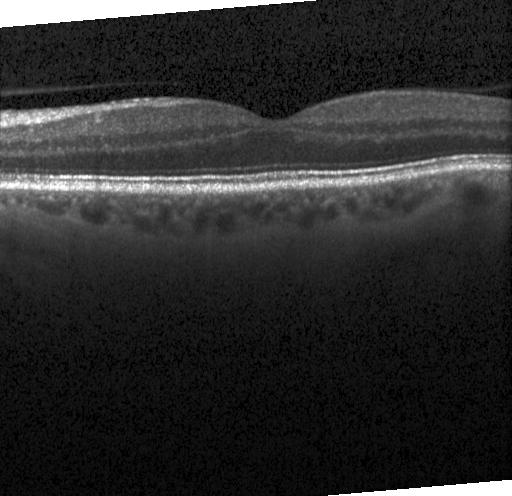

Heidelberg Spectralis · optical coherence tomography B-scan · horizontal scan through the fovea — Finding: no evidence of CNV, DME, or drusen.